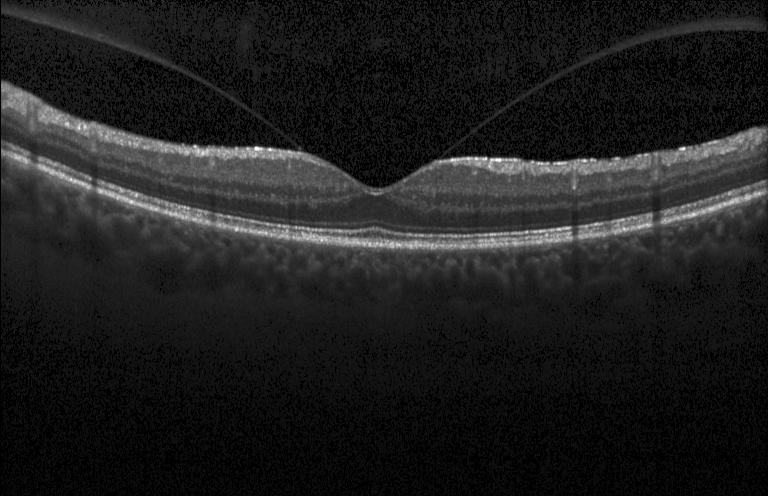 Spectral-domain optical coherence tomography; optical coherence tomography B-scan — No CNV, no DME, and no drusen.